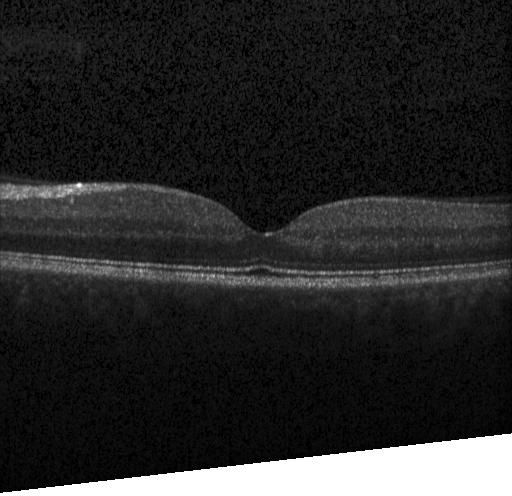 Retinal OCT cross-section showing no evidence of choroidal neovascularization, diabetic macular edema, or drusen.